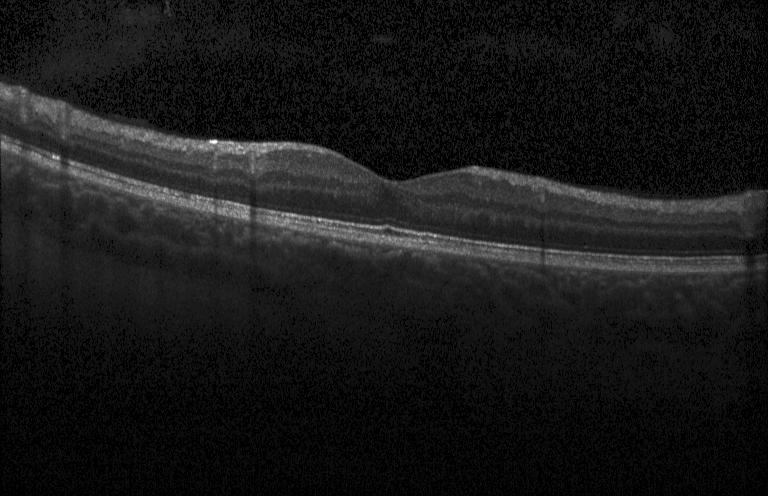

Retinal OCT B-scan. Assessment: no CNV, DME, or drusen.